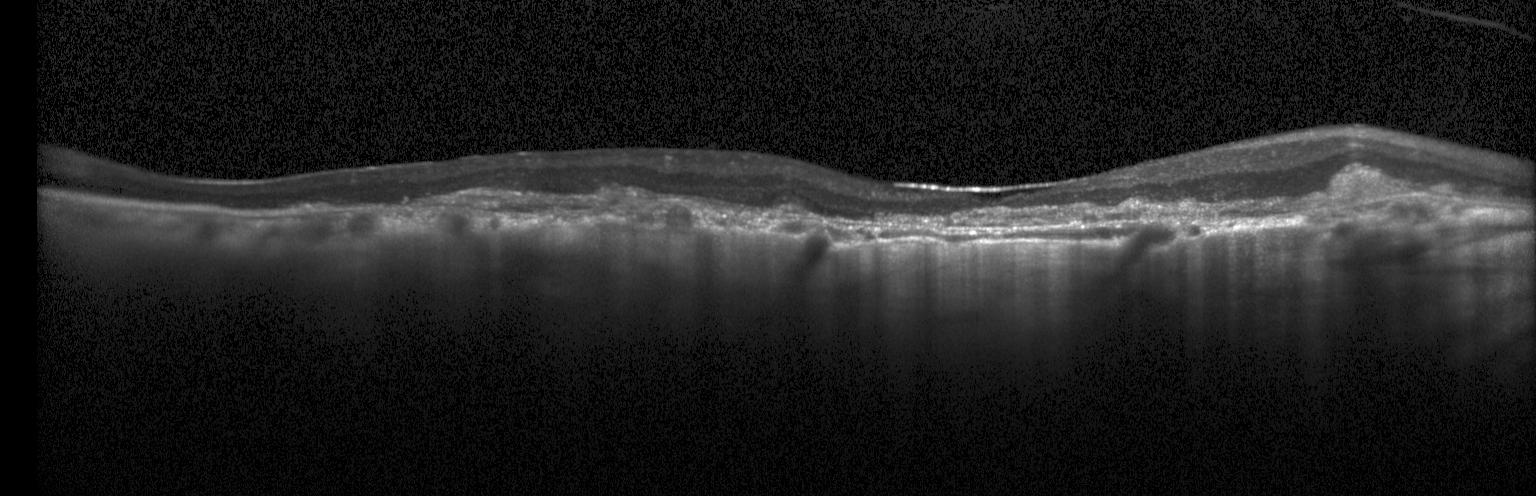
OCT line scan. Finding: a choroidal neovascular membrane.